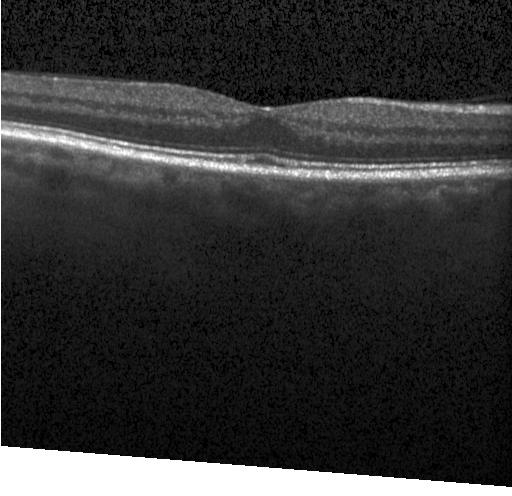 Optical coherence tomography B-scan; spectral-domain OCT; instrument: Heidelberg Spectralis — This B-scan demonstrates no choroidal neovascularization, no diabetic macular edema, and no drusen.